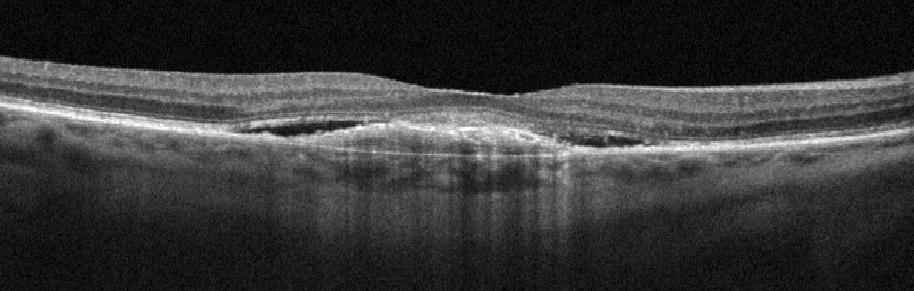
Optical coherence tomography scan. Oculus dexter
OCT finding: age-related macular degeneration (AMD).